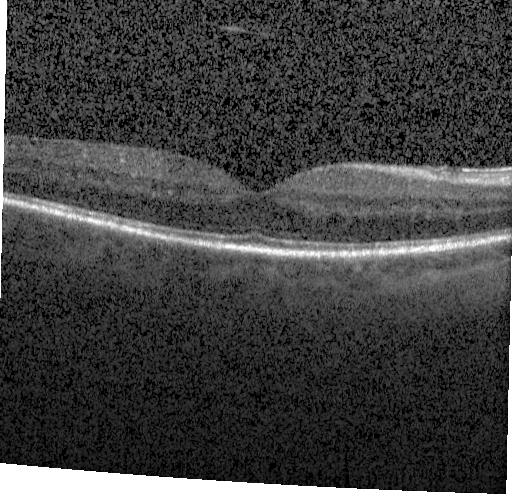 Centered on the fovea. Heidelberg Spectralis OCT system. Retinal OCT cross-section. Macular OCT: no choroidal neovascularization, diabetic macular edema, or drusen.